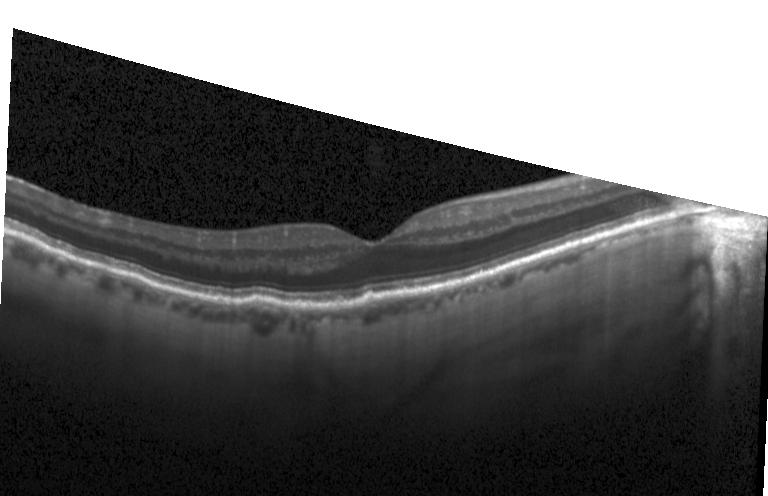

Spectral-domain OCT; Heidelberg Spectralis; horizontal scan through the fovea; retinal OCT cross-section.
The scan shows multiple drusen.